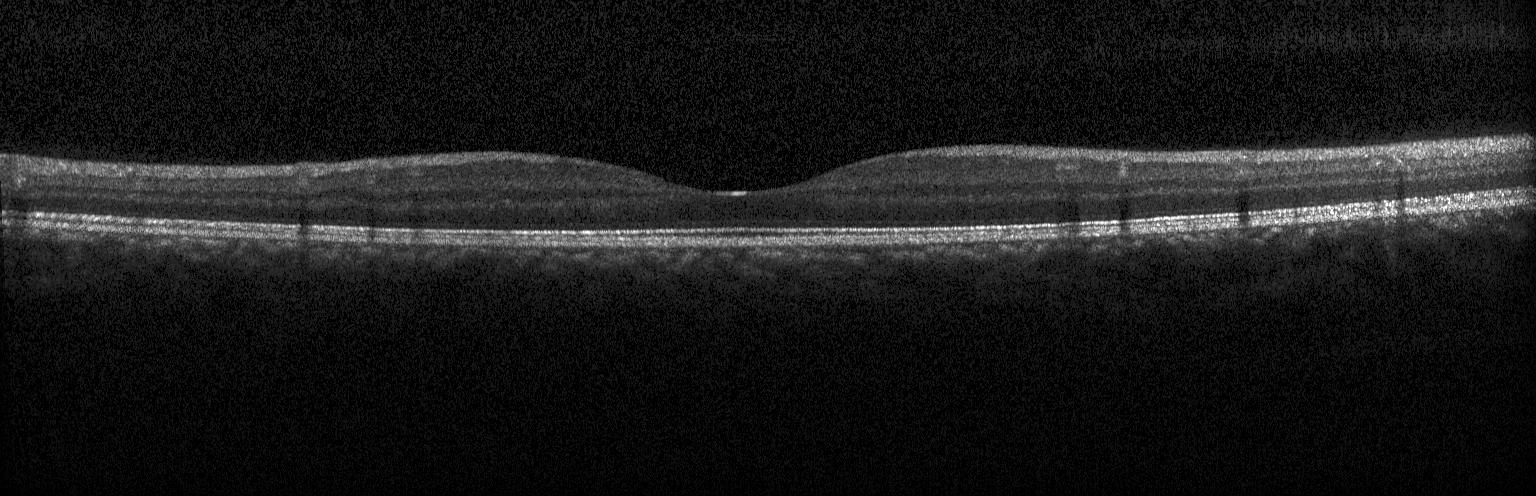 OCT scan showing no choroidal neovascularization, diabetic macular edema, or drusen.